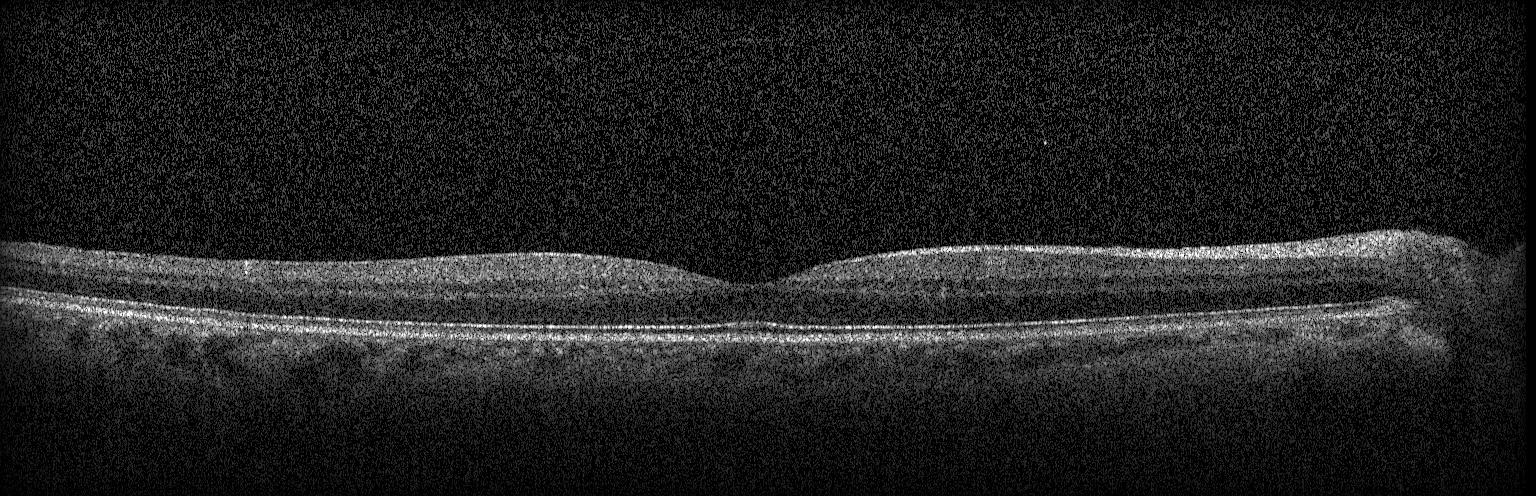
OCT B-scan — OCT finding: no choroidal neovascularization, diabetic macular edema, or drusen.